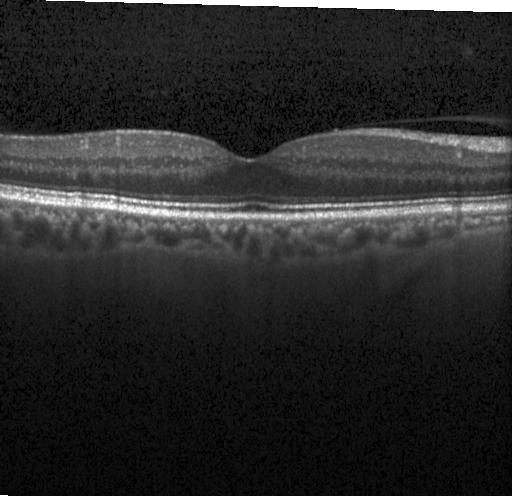

Optical coherence tomography scan. Diagnosis: no evidence of choroidal neovascularization, diabetic macular edema, or drusen.